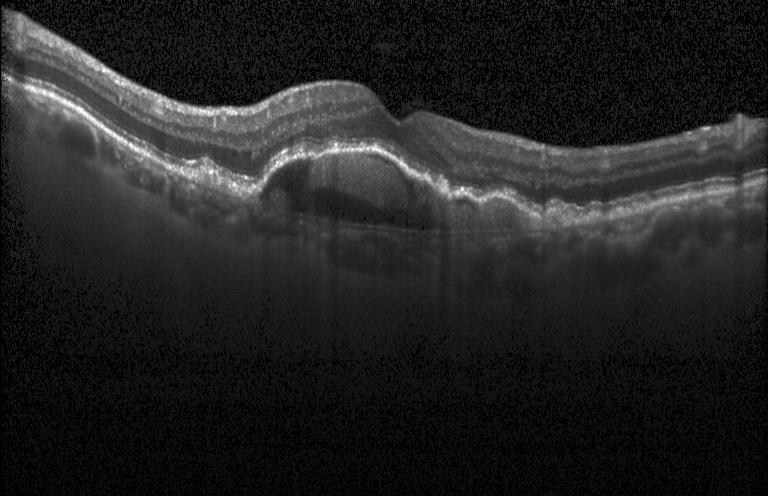

Centered on the fovea. Spectral-domain OCT. Optical coherence tomography B-scan — Finding: multiple drusen.